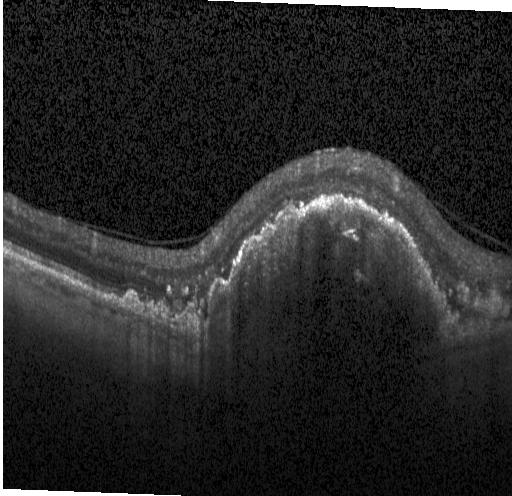

Impression: a choroidal neovascular membrane.